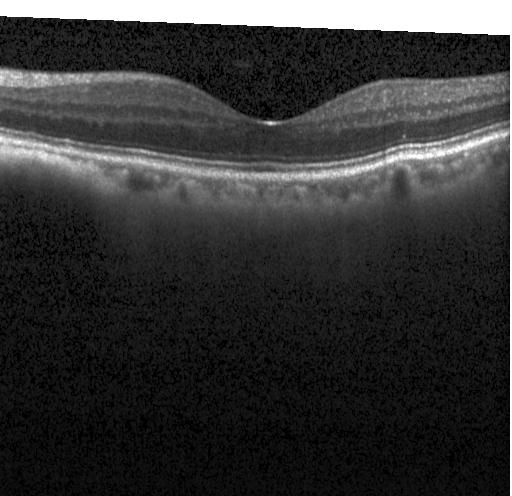
Retinal OCT cross-section, acquired on a Heidelberg Spectralis — This B-scan demonstrates no choroidal neovascularization, no diabetic macular edema, and no drusen.